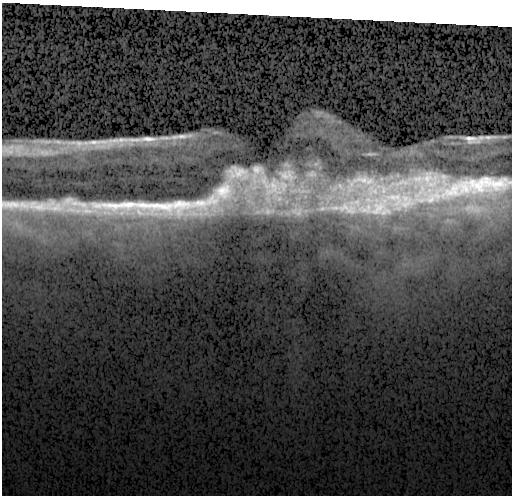
Retinal OCT cross-section
Impression: CNV.